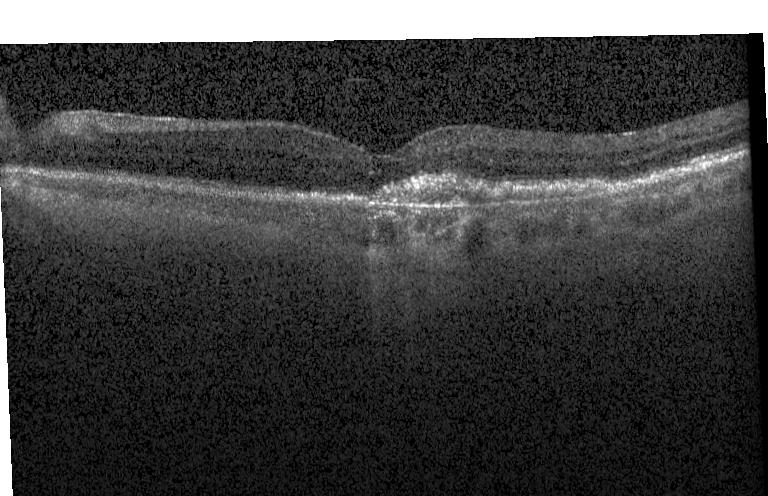

Optical coherence tomography B-scan — Choroidal neovascularization.